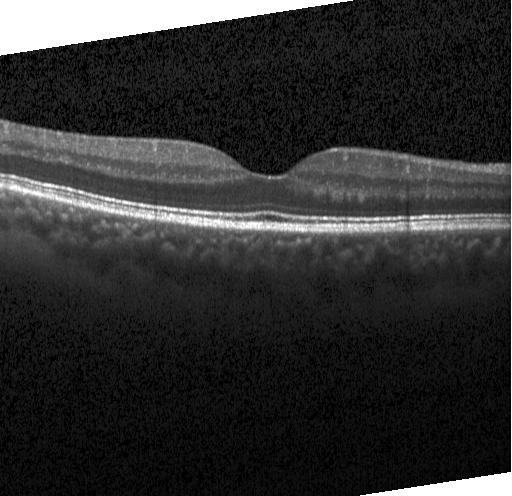
Retinal OCT cross-section · instrument: Heidelberg Spectralis · spectral-domain optical coherence tomography · centered on the fovea — Macular OCT: no CNV, no DME, and no drusen.